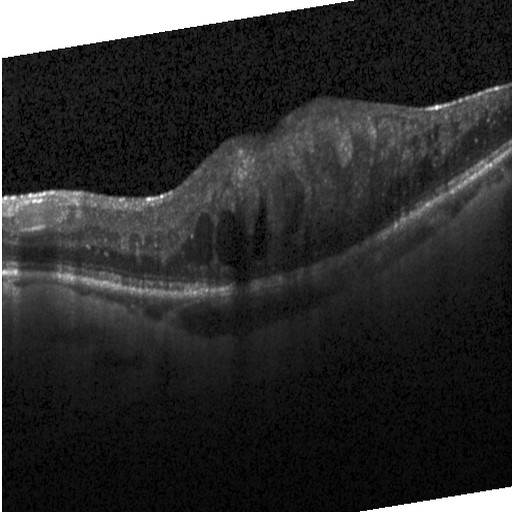
Retinal OCT cross-section showing diabetic macular edema.